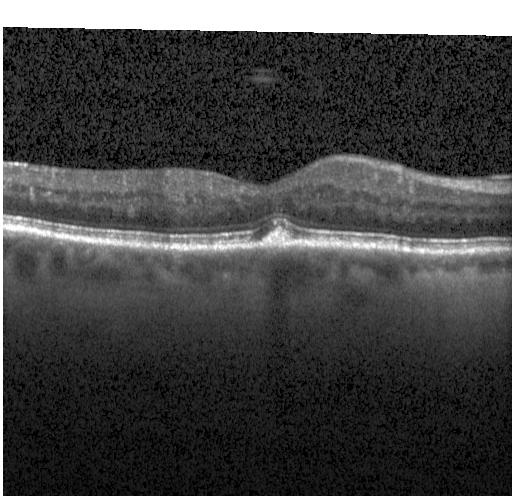 Diagnosis: sub-RPE drusenoid deposits.